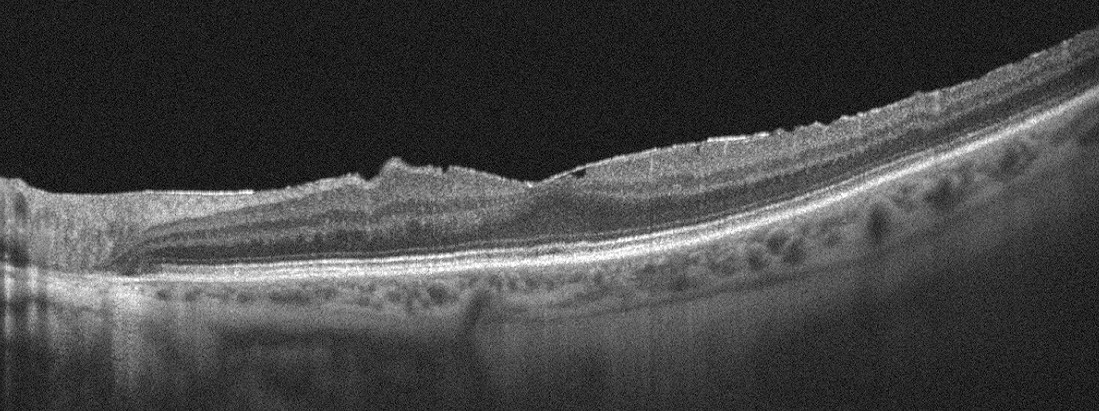 Retinal OCT cross-section; instrument: Optovue Avanti RTVue XR
This B-scan demonstrates ERM.